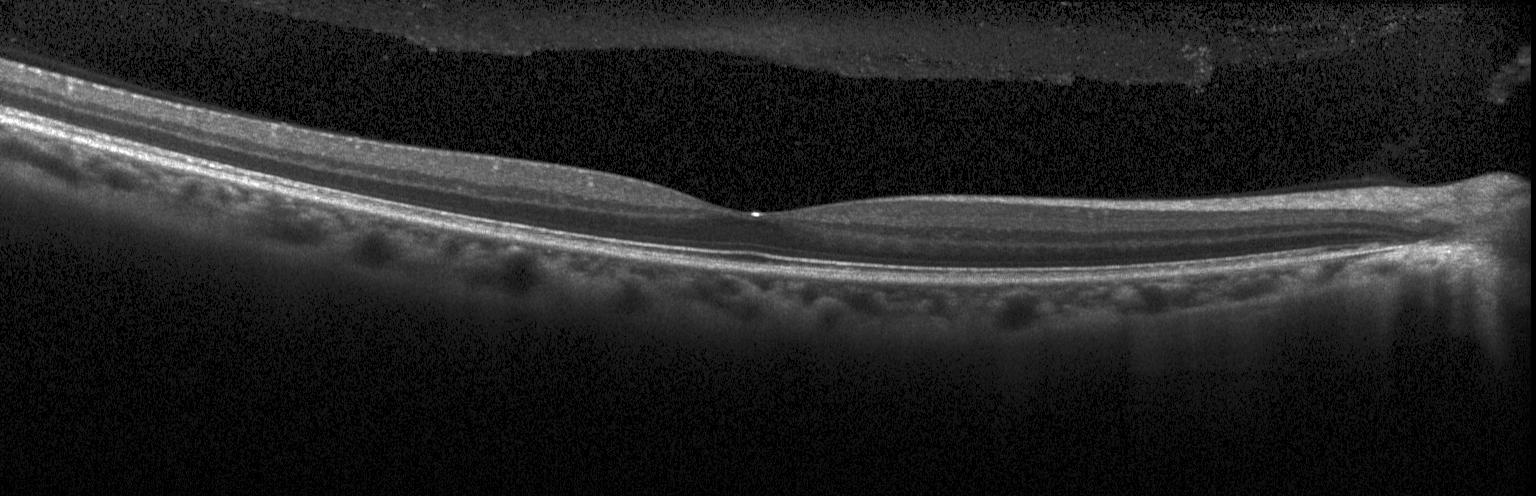
OCT B-scan showing no evidence of choroidal neovascularization, diabetic macular edema, or drusen.